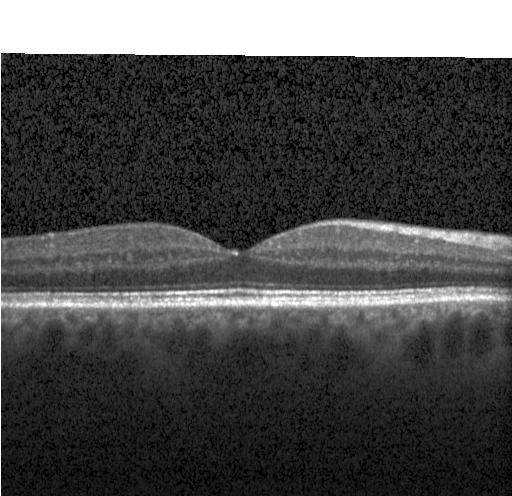 Optical coherence tomography B-scan. Fovea-centered. Instrument: Heidelberg Spectralis
Finding: no CNV, no DME, and no drusen.